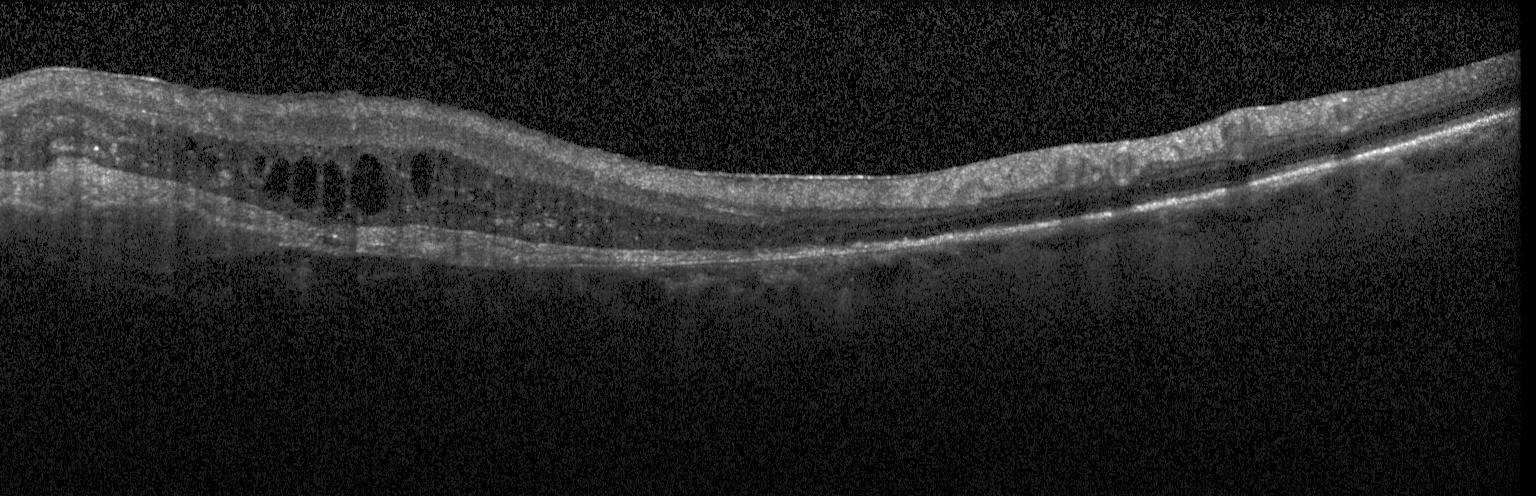

Retinal OCT cross-section, Heidelberg Spectralis OCT system, fovea-centered — Finding: choroidal neovascularization.